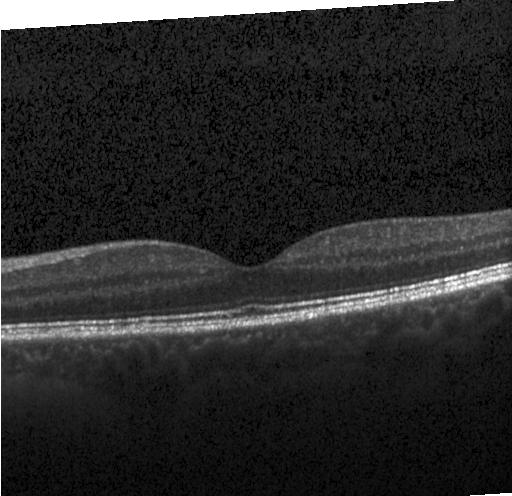

Optical coherence tomography scan. Assessment: no evidence of CNV, DME, or drusen.